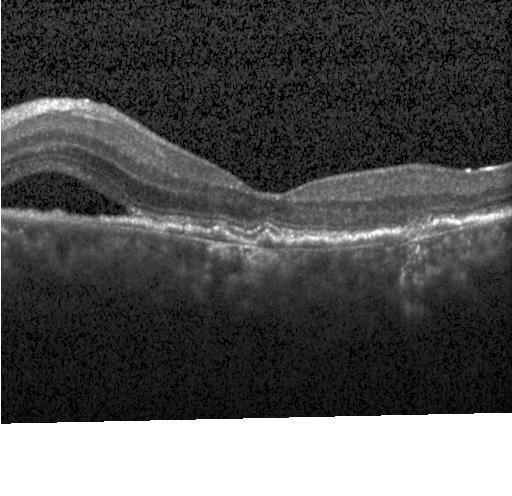

Through the macula. Retinal OCT B-scan. SD-OCT. A choroidal neovascular membrane.